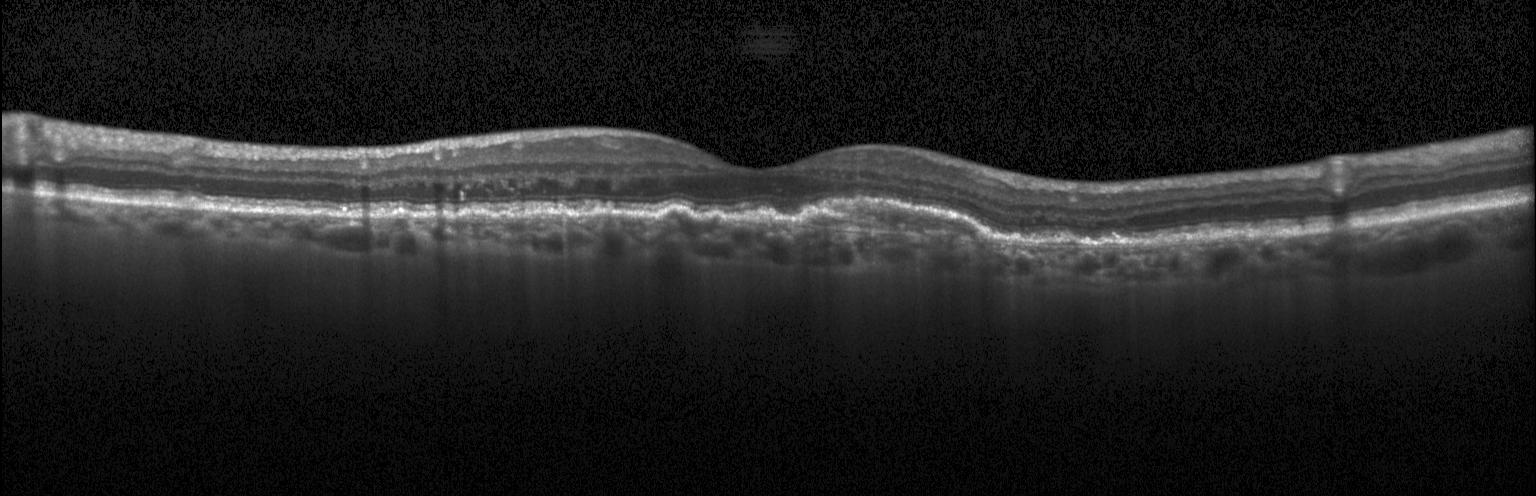 Retinal OCT cross-section. Macular scan. SD-OCT — The scan shows a choroidal neovascular membrane.